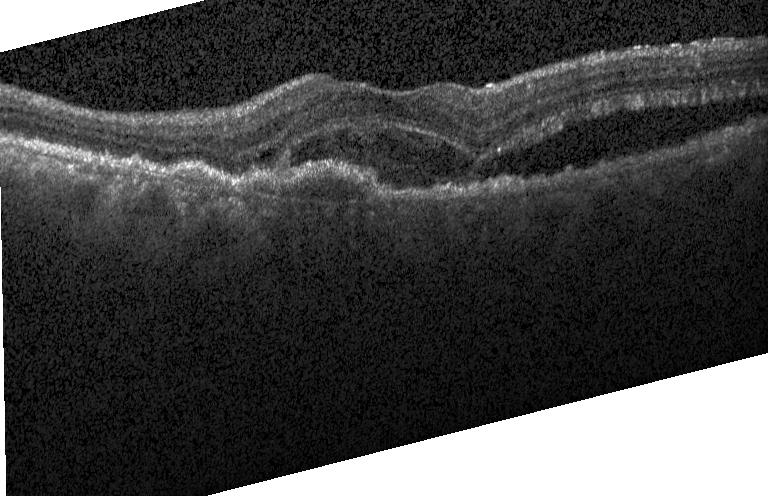 OCT B-scan · spectral-domain OCT · instrument: Heidelberg Spectralis.
This B-scan demonstrates a choroidal neovascular membrane.